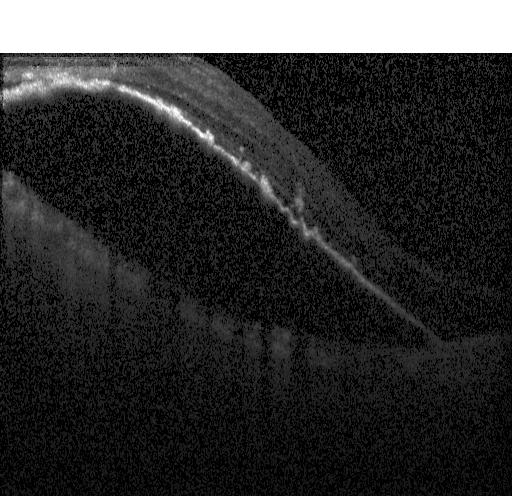

Optical coherence tomography scan, Heidelberg Spectralis OCT system, spectral-domain optical coherence tomography.
Assessment: CNV.